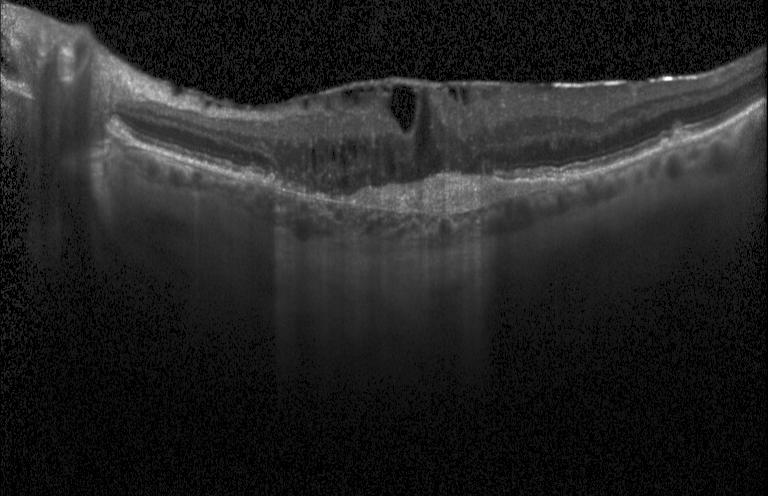
Heidelberg Spectralis OCT system, fovea-centered, OCT line scan, spectral-domain optical coherence tomography.
The scan shows CNV.